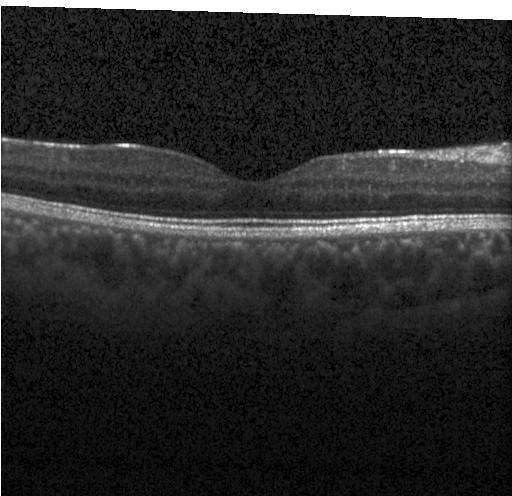 Heidelberg Spectralis OCT system; spectral-domain OCT; OCT B-scan; fovea-centered
Impression: neither choroidal neovascularization, diabetic macular edema, nor drusen.